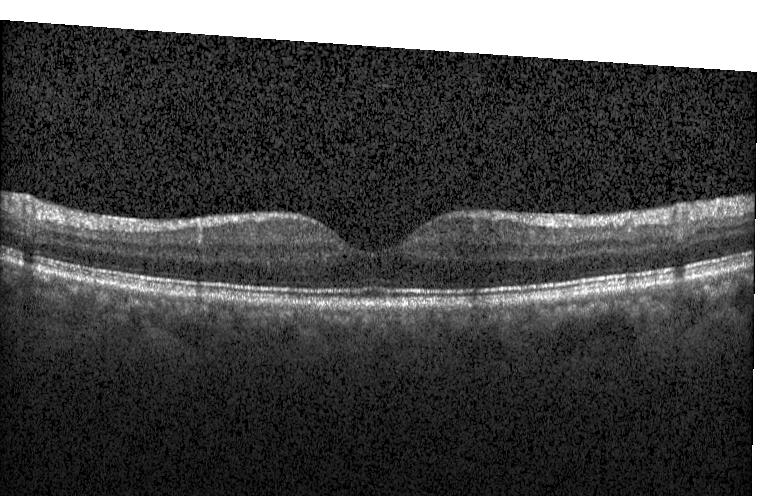

OCT B-scan; acquired on a Heidelberg Spectralis; through the macula
Diagnosis: no evidence of choroidal neovascularization, diabetic macular edema, or drusen.